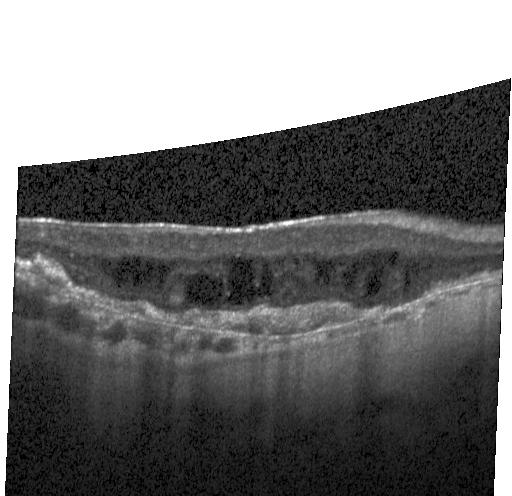
SD-OCT; retinal OCT cross-section — Choroidal neovascularization.